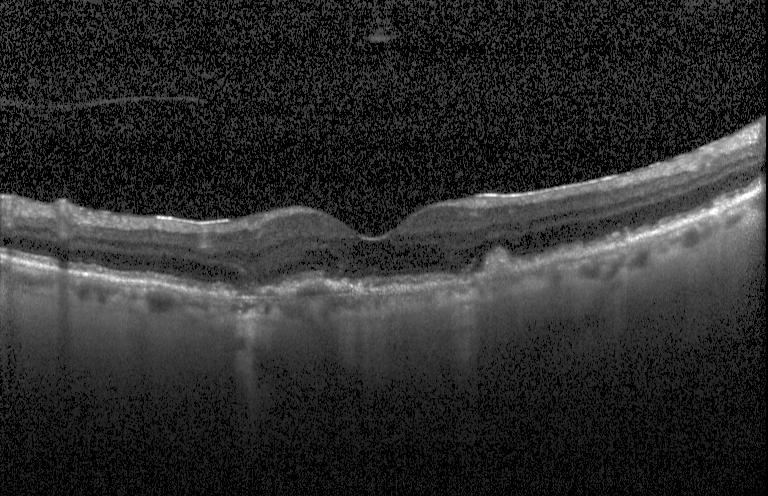
OCT line scan
Finding: a choroidal neovascular membrane.